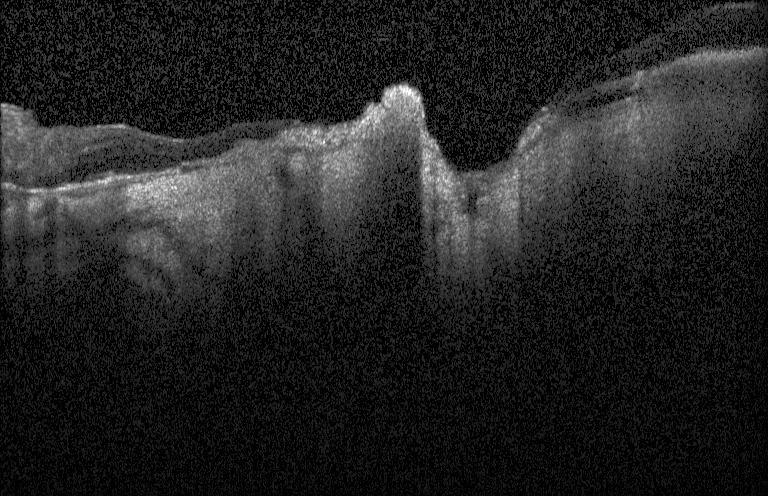

A choroidal neovascular membrane.